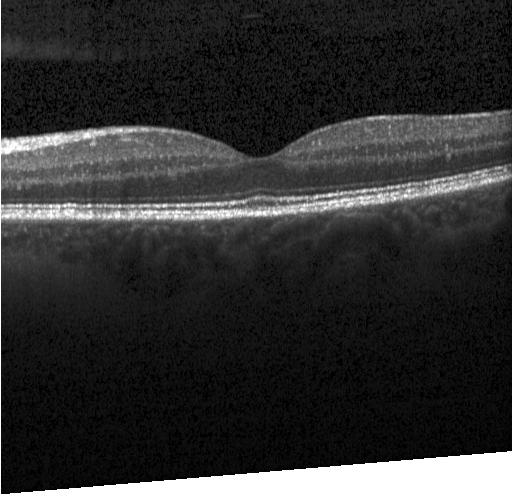 Finding: neither choroidal neovascularization, diabetic macular edema, nor drusen.